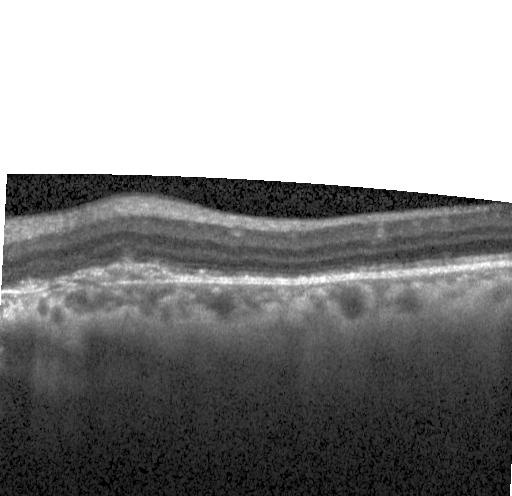

Diagnosis: choroidal neovascularization (CNV).